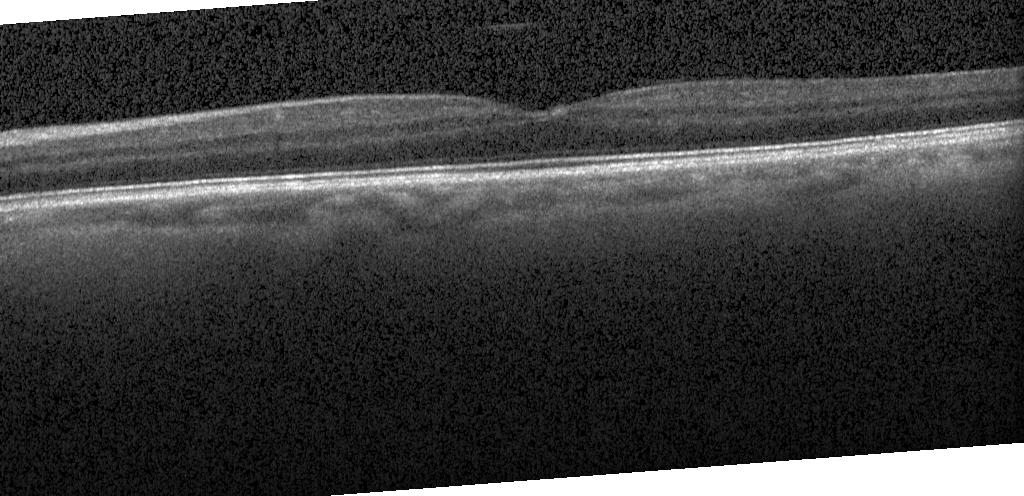
Optical coherence tomography B-scan. Instrument: Heidelberg Spectralis. Spectral-domain optical coherence tomography. Dx: neither choroidal neovascularization, diabetic macular edema, nor drusen.